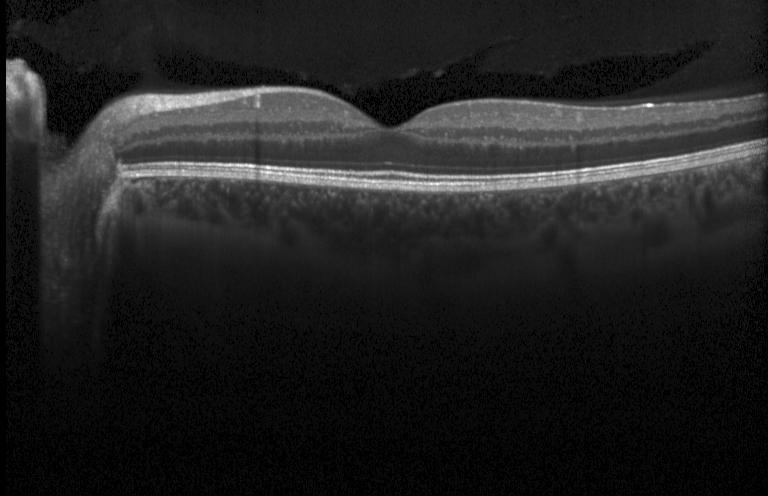 Optical coherence tomography scan · spectral-domain optical coherence tomography · instrument: Heidelberg Spectralis. Diagnosis: no choroidal neovascularization, diabetic macular edema, or drusen.